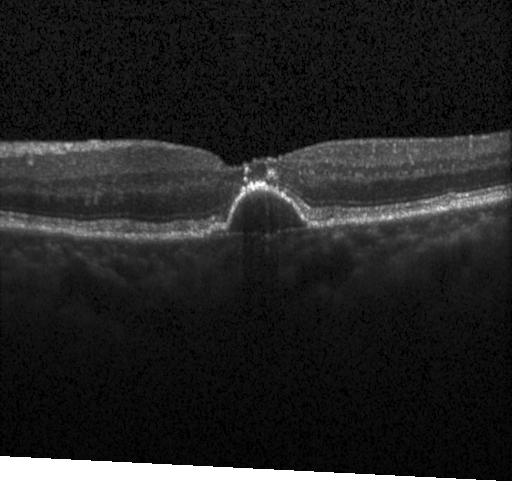
OCT line scan — Impression: choroidal neovascularization (CNV).